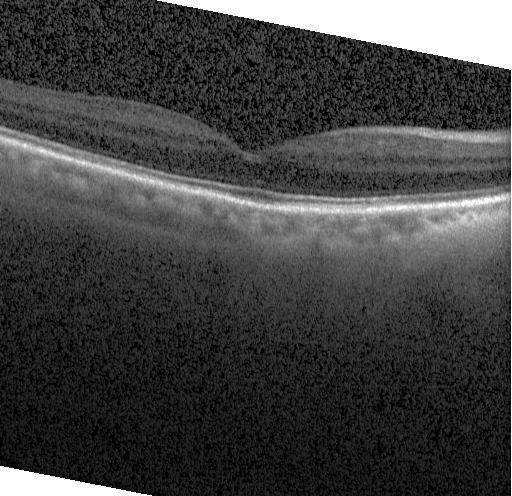
OCT line scan; horizontal scan through the fovea; instrument: Heidelberg Spectralis; spectral-domain optical coherence tomography — The scan shows no CNV, no DME, and no drusen.